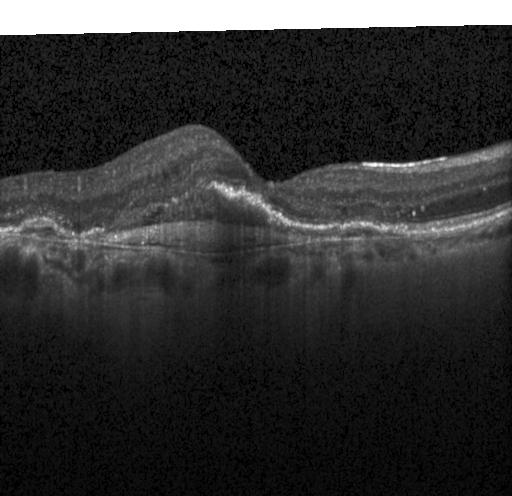 Retinal OCT cross-section
Finding: a choroidal neovascular membrane.